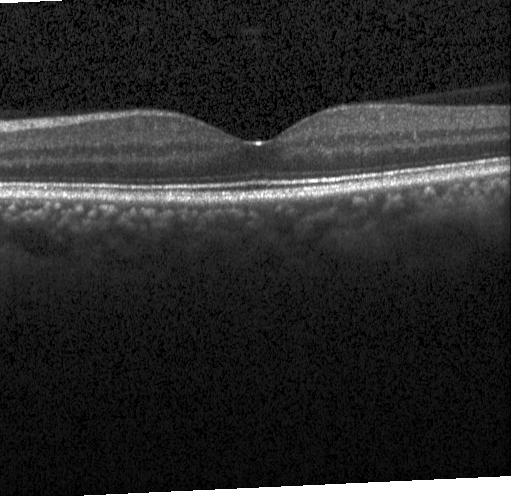
Macular OCT: no CNV, no DME, and no drusen.